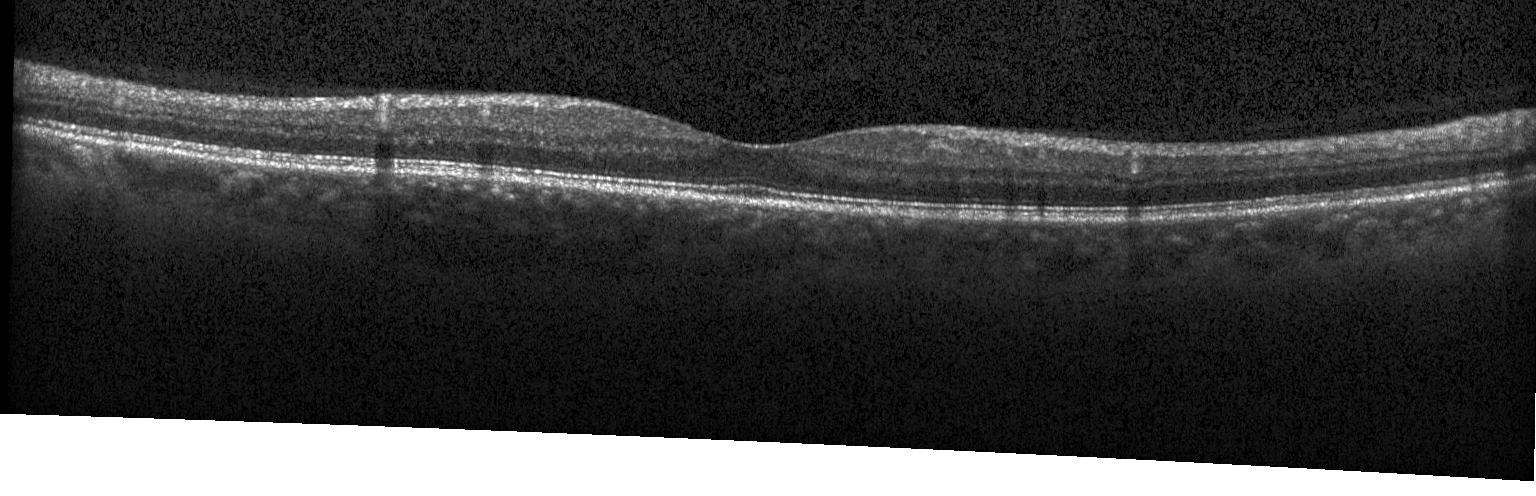 Through the macula, acquired on a Heidelberg Spectralis, retinal OCT cross-section. Finding: neither choroidal neovascularization, diabetic macular edema, nor drusen.